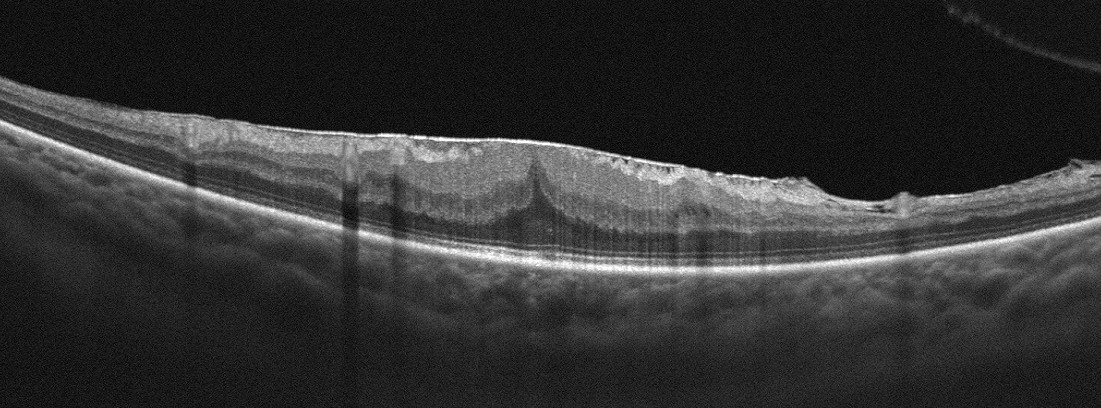 Fovea-centered; instrument: Optovue Avanti RTVue XR; retinal OCT B-scan — Finding: epiretinal membrane (ERM).